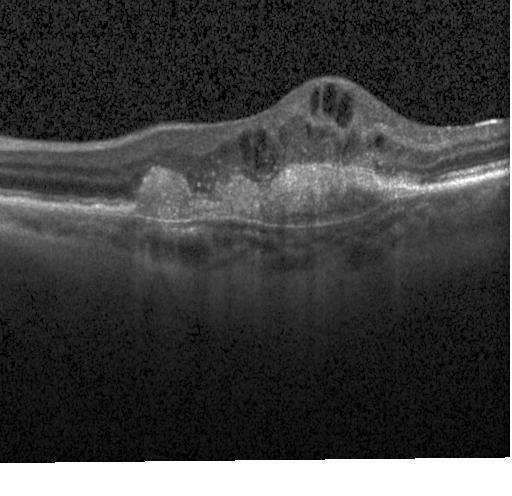

This B-scan demonstrates CNV.